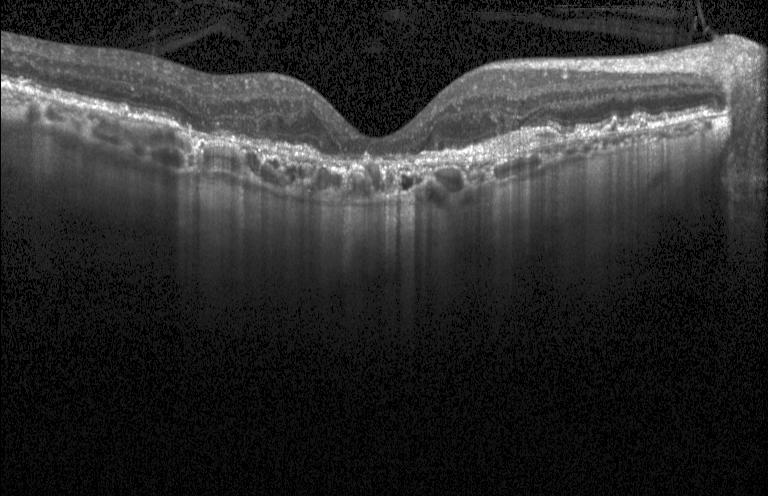
Retinal OCT B-scan. Assessment: a choroidal neovascular membrane.